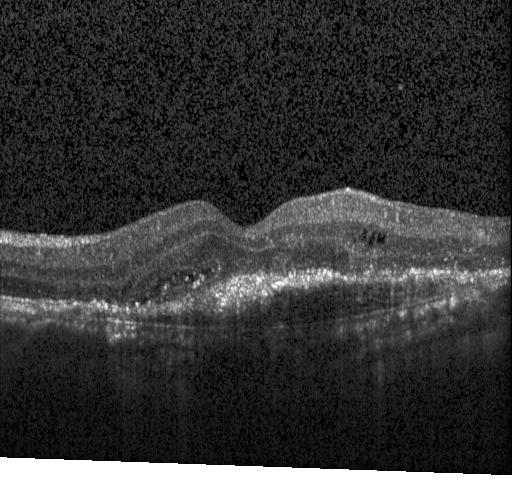
OCT line scan.
A choroidal neovascular membrane.